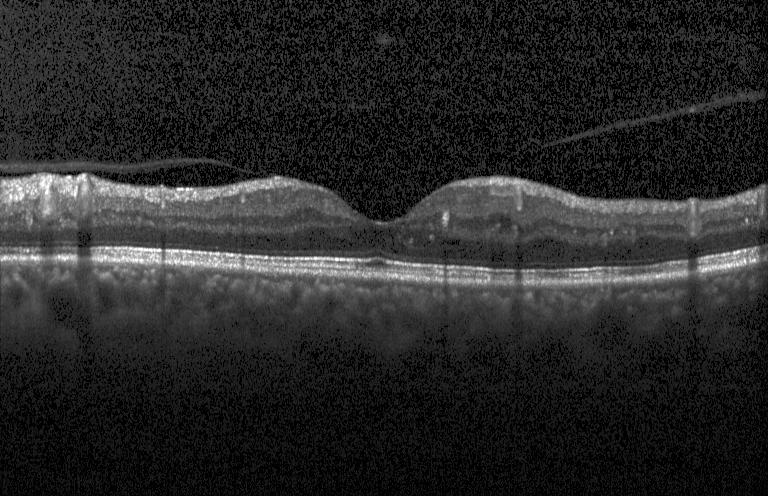
Spectral-domain optical coherence tomography. Optical coherence tomography B-scan. Dx: DME.